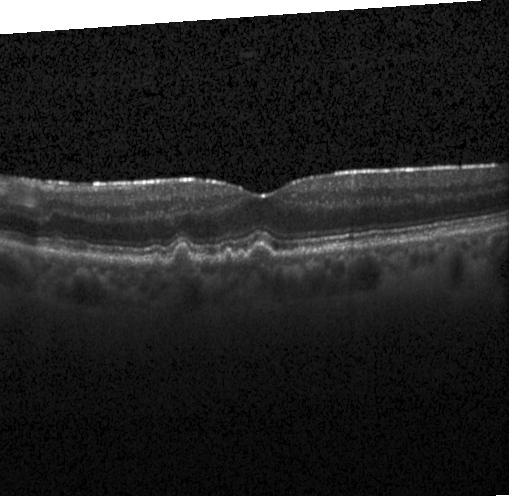 Acquired on a Heidelberg Spectralis. Spectral-domain optical coherence tomography. Retinal OCT B-scan — Diagnosis: multiple drusen.